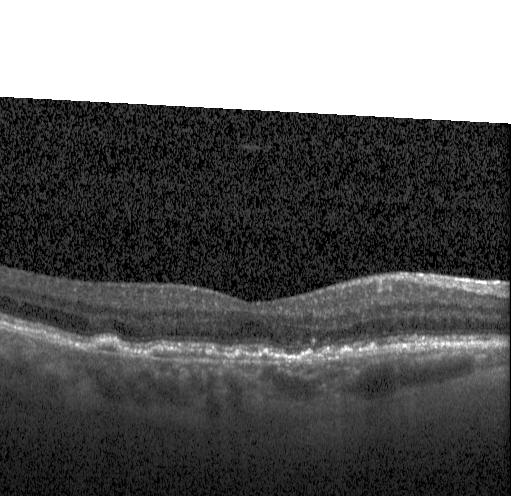
OCT scan showing a choroidal neovascular membrane.